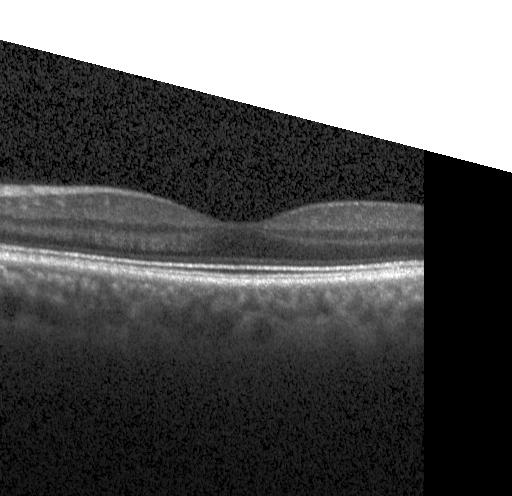

Retinal OCT cross-section showing no evidence of CNV, DME, or drusen.